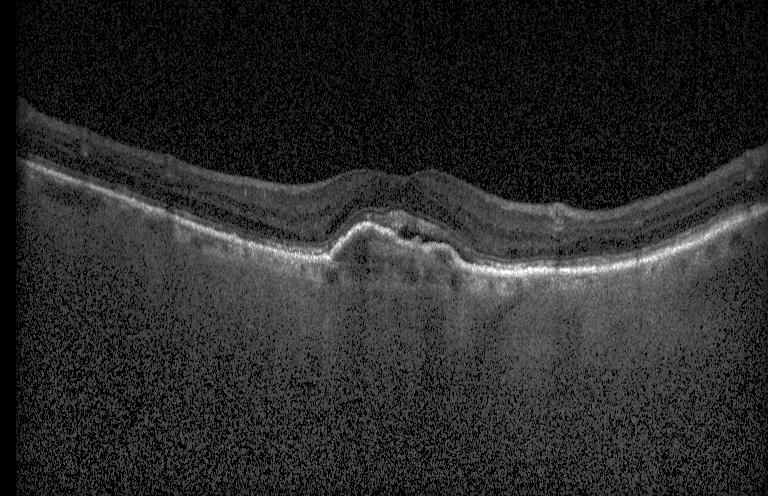
OCT line scan · Heidelberg Spectralis — Diagnosis: choroidal neovascularization (CNV).